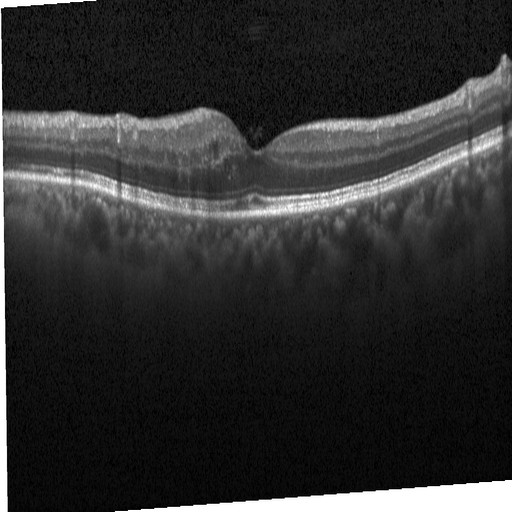

Retinal OCT cross-section showing diabetic macular edema.